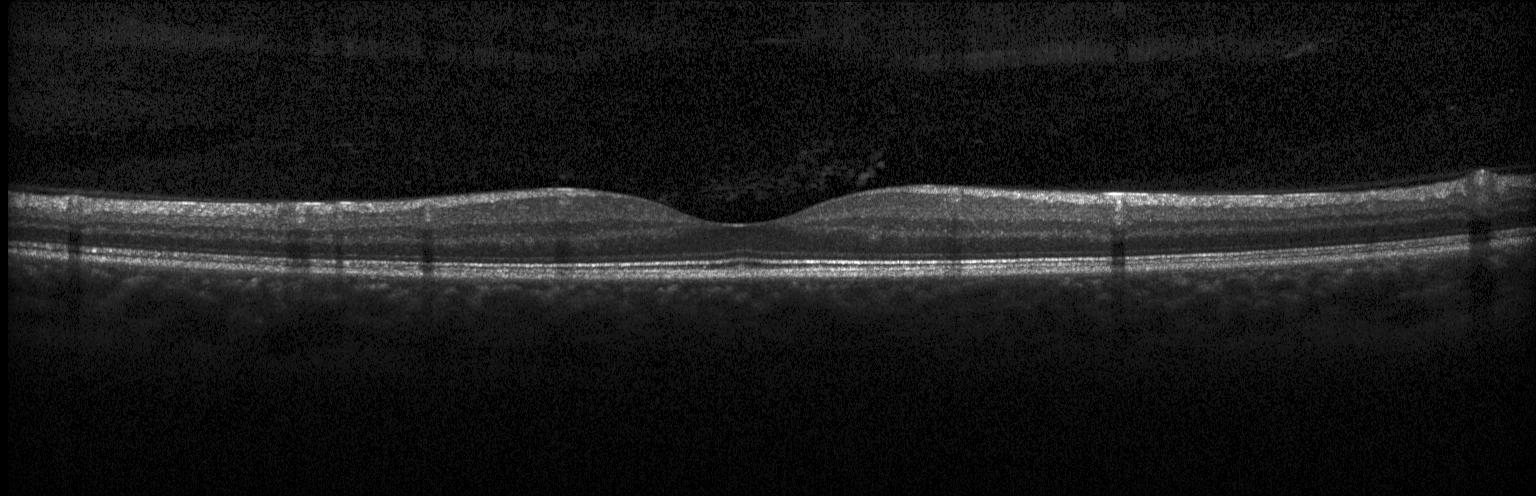
Acquired on a Heidelberg Spectralis, spectral-domain OCT, OCT B-scan. Dx: neither choroidal neovascularization, diabetic macular edema, nor drusen.